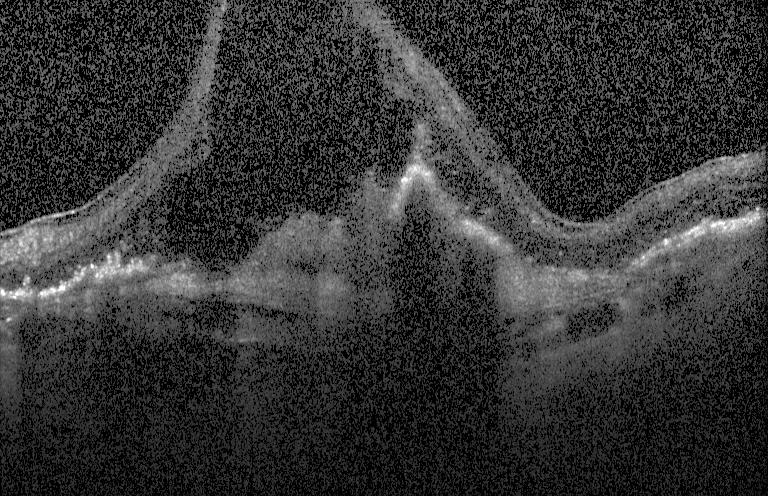

Optical coherence tomography scan — Impression: a choroidal neovascular membrane.